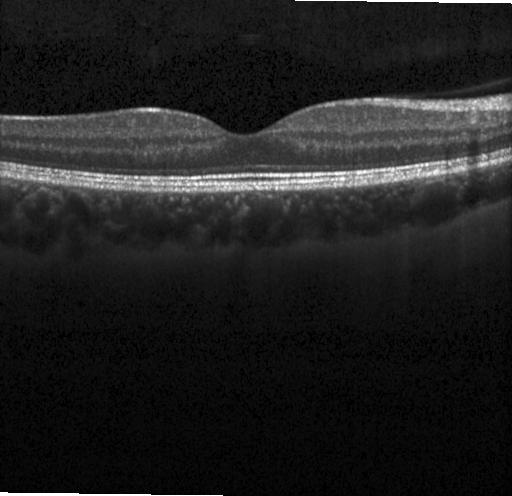 Diagnosis: no choroidal neovascularization, no diabetic macular edema, and no drusen.